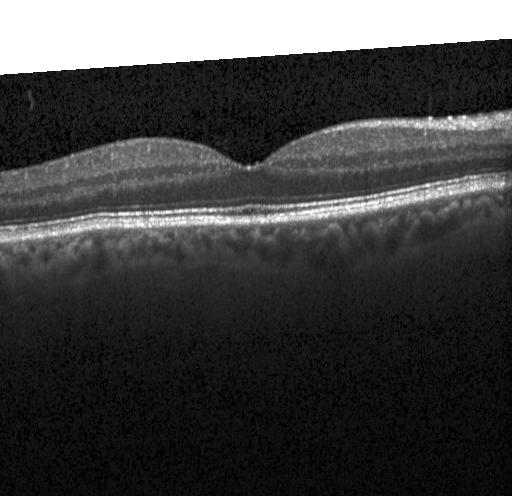

Instrument: Heidelberg Spectralis · retinal OCT cross-section. This B-scan demonstrates neither choroidal neovascularization, diabetic macular edema, nor drusen.